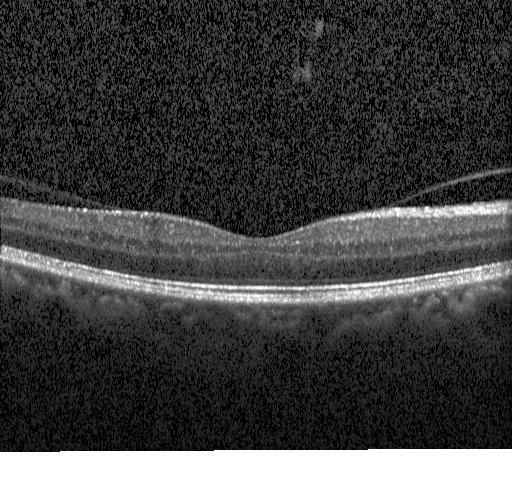
Optical coherence tomography scan.
Diagnosis: neither CNV, DME, nor drusen.